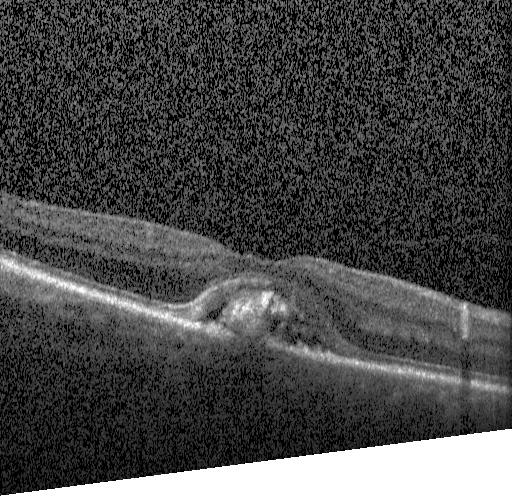 Optical coherence tomography scan, centered on the fovea — Macular OCT: choroidal neovascularization.